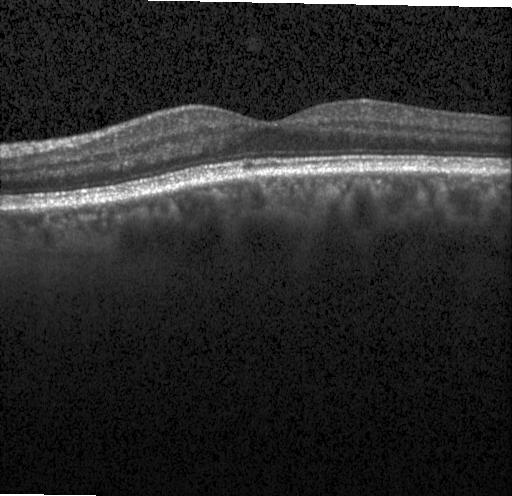 Retinal OCT B-scan, Heidelberg Spectralis — Impression: no CNV, no DME, and no drusen.